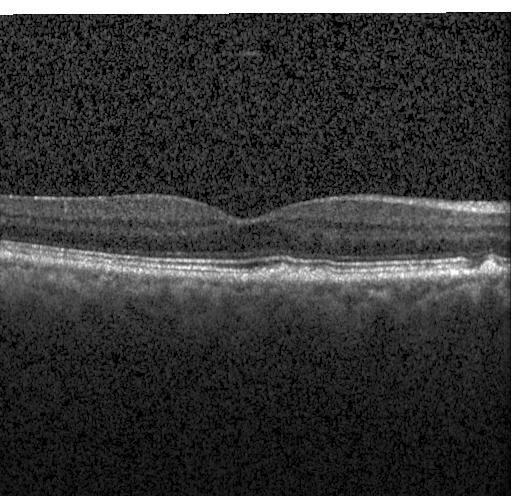
Optical coherence tomography B-scan, instrument: Heidelberg Spectralis, macular scan, SD-OCT
OCT finding: sub-RPE drusenoid deposits.